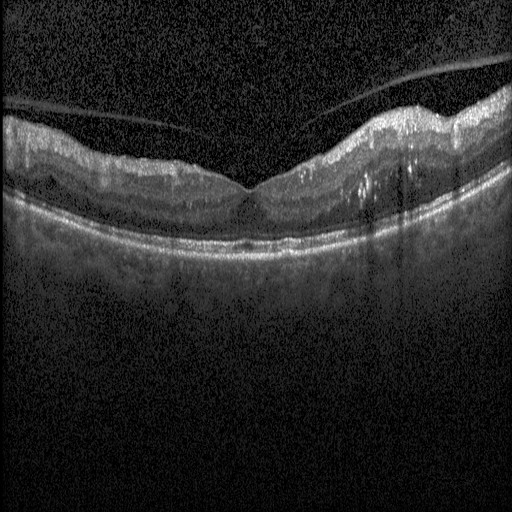 Finding: diabetic macular edema (DME).